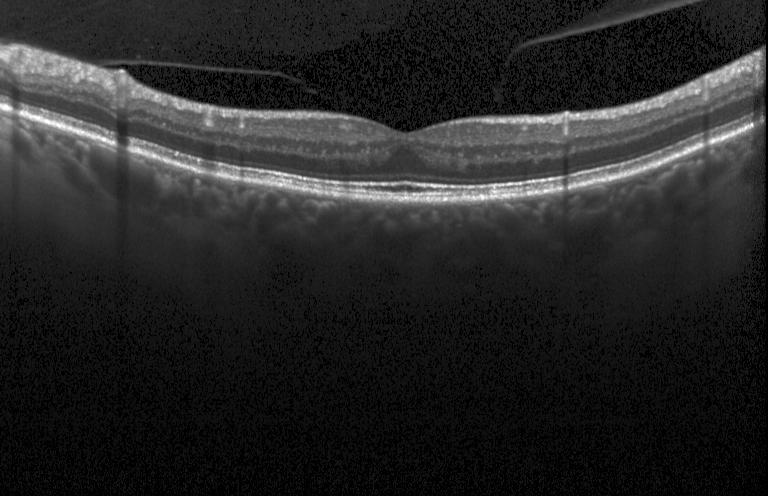
Retinal OCT B-scan
No choroidal neovascularization, diabetic macular edema, or drusen.